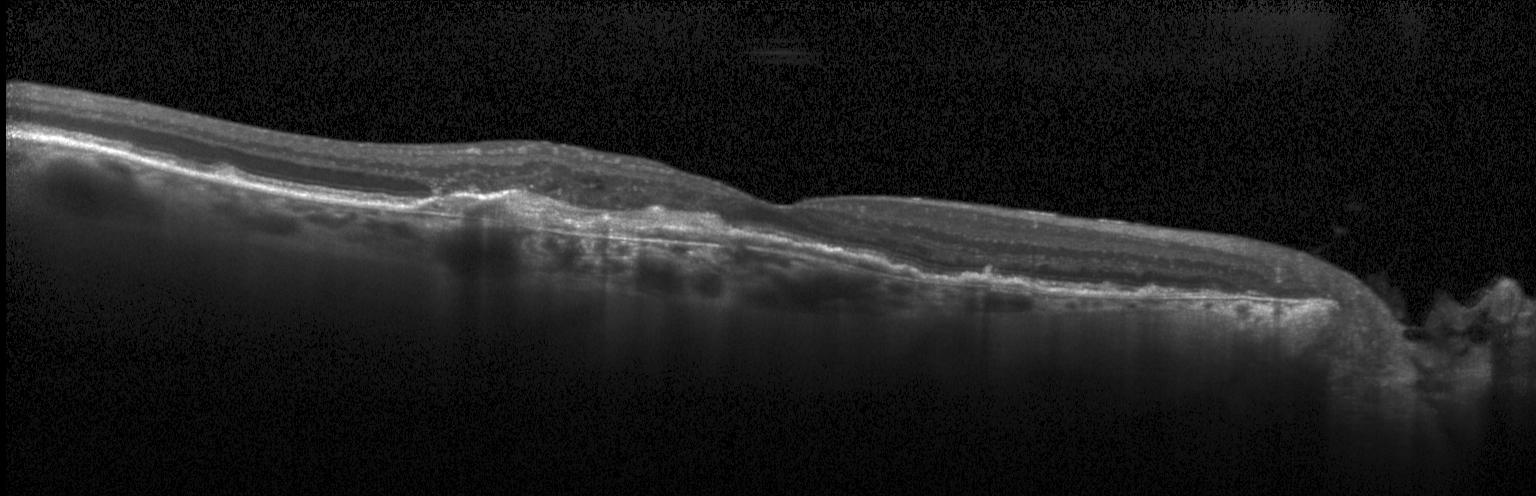

Retinal OCT cross-section
Finding: choroidal neovascularization (CNV).